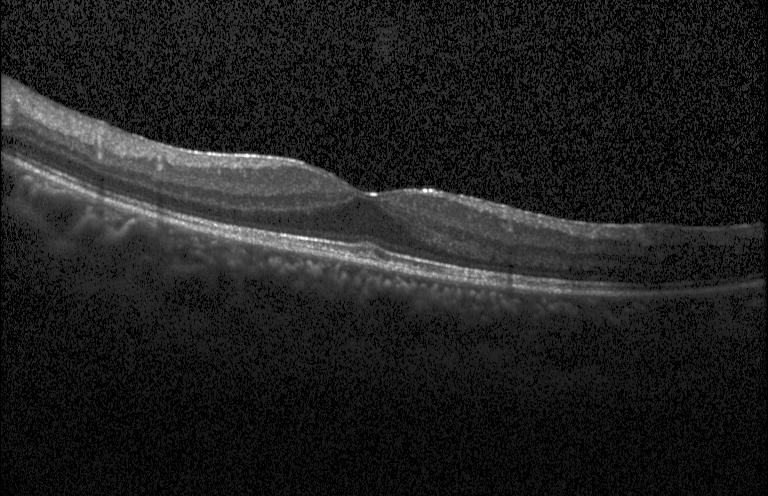 OCT B-scan, Heidelberg Spectralis OCT system, centered on the fovea, SD-OCT.
Finding: no evidence of choroidal neovascularization, diabetic macular edema, or drusen.